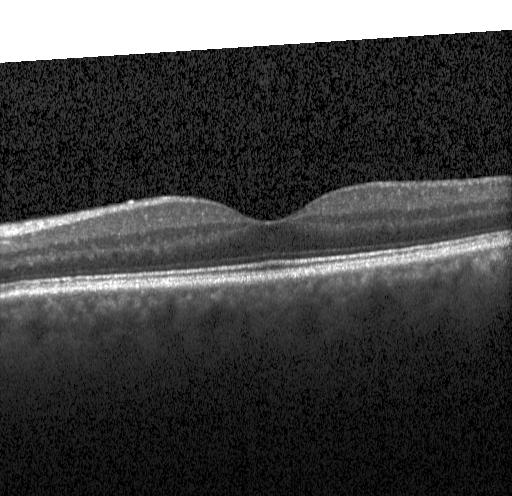
OCT finding: no choroidal neovascularization, no diabetic macular edema, and no drusen.